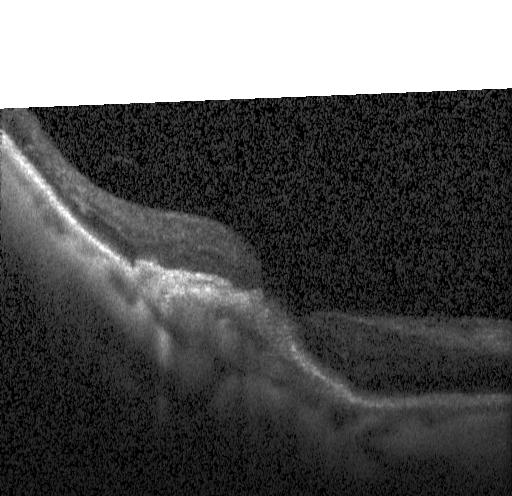
This B-scan demonstrates a choroidal neovascular membrane.